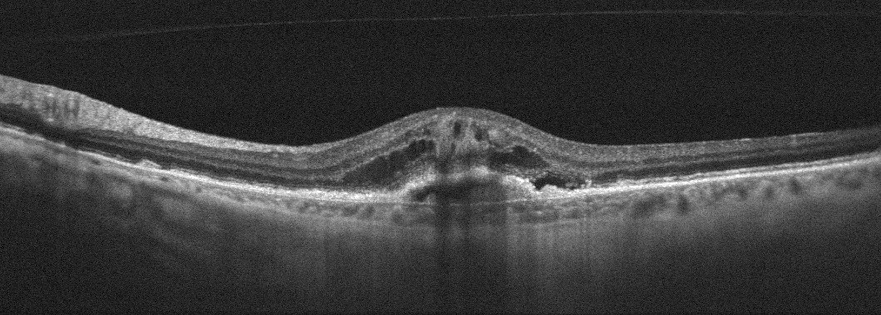
Spectral-domain OCT B-scan: AMD.